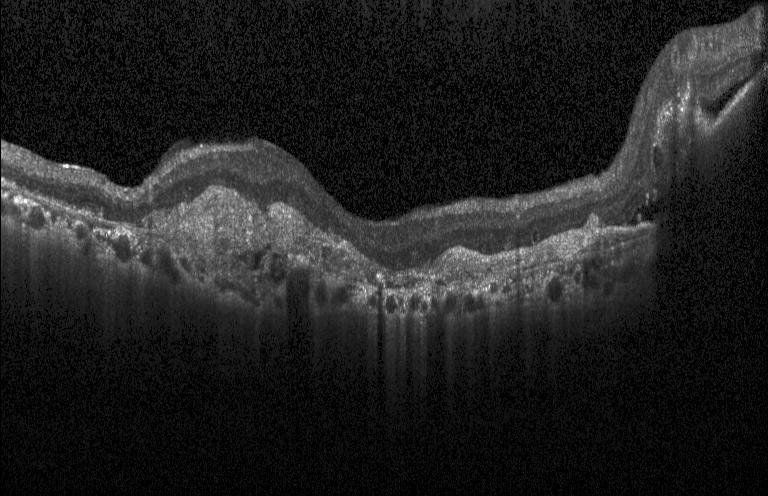 Retinal OCT cross-section — Assessment: choroidal neovascularization.